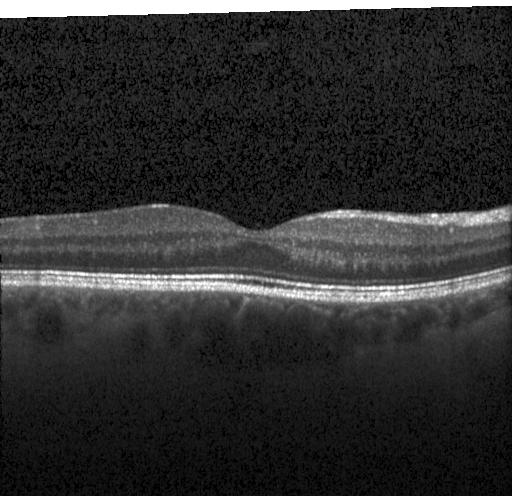 Finding: no choroidal neovascularization, diabetic macular edema, or drusen.